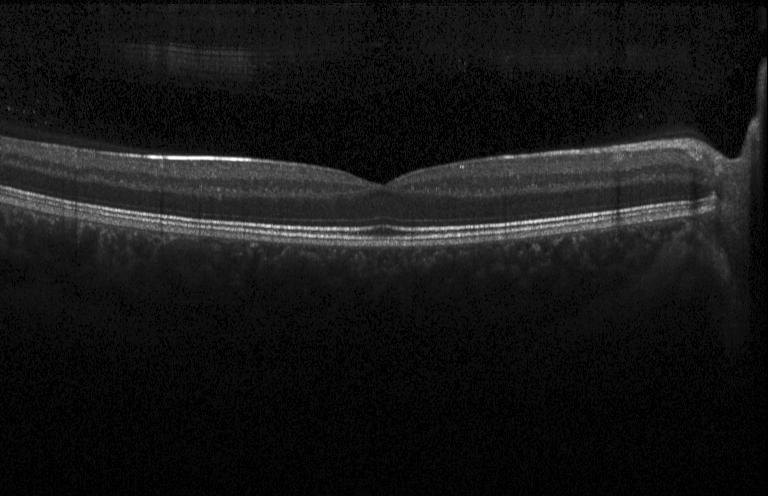 OCT B-scan. Heidelberg Spectralis OCT system. Finding: no evidence of choroidal neovascularization, diabetic macular edema, or drusen.